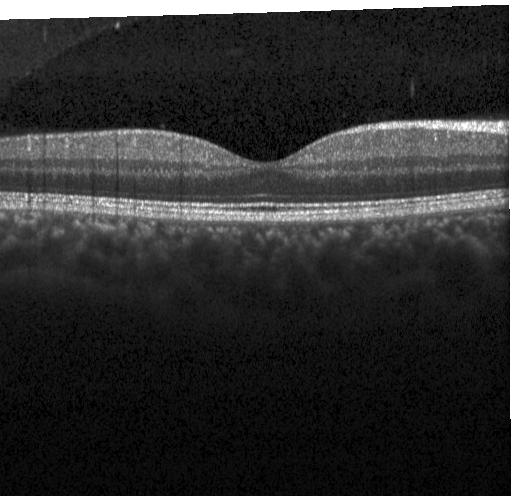
OCT finding: no choroidal neovascularization, no diabetic macular edema, and no drusen.